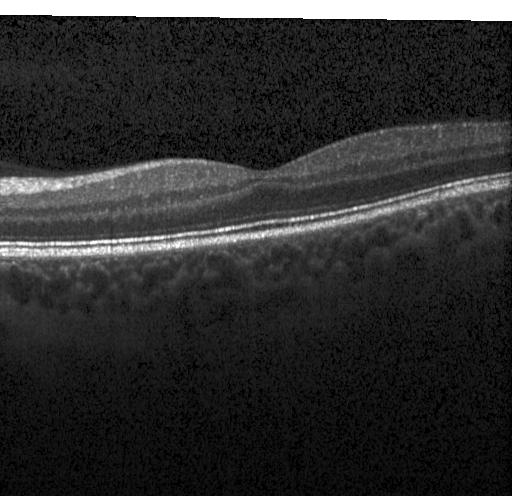
Instrument: Heidelberg Spectralis. Through the macula. Optical coherence tomography B-scan
Impression: no evidence of choroidal neovascularization, diabetic macular edema, or drusen.